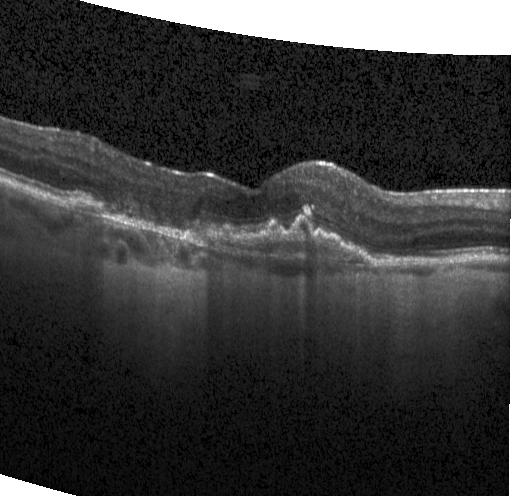

Diagnosis: choroidal neovascularization.